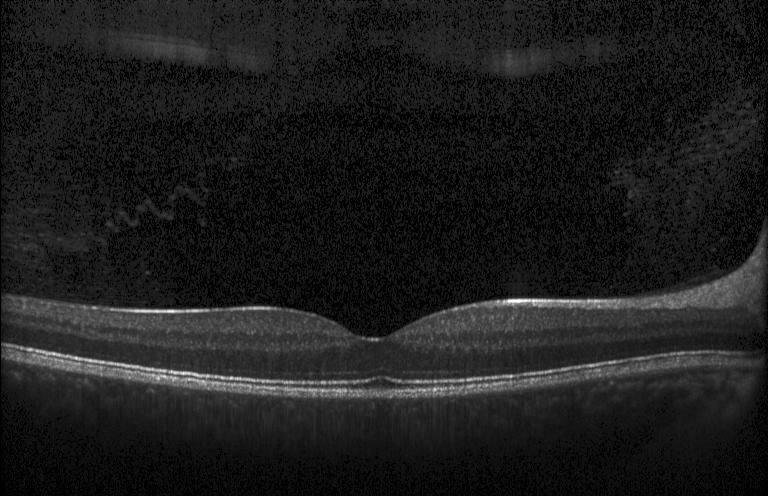
Macular OCT: no evidence of choroidal neovascularization, diabetic macular edema, or drusen.